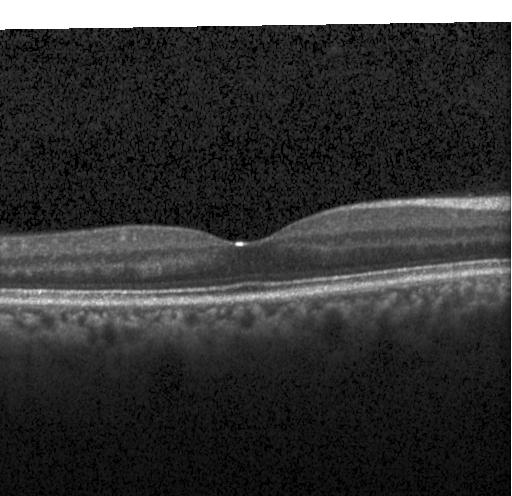

Optical coherence tomography B-scan, Heidelberg Spectralis, SD-OCT
Neither choroidal neovascularization, diabetic macular edema, nor drusen.